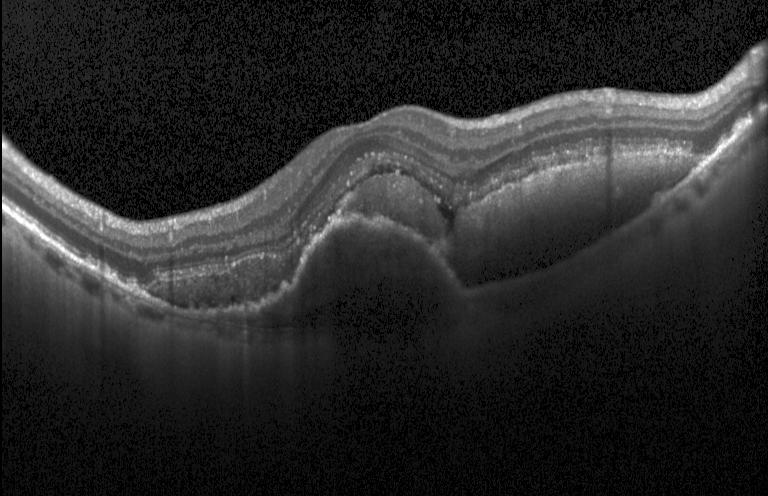 Spectral-domain optical coherence tomography; Heidelberg Spectralis; fovea-centered; optical coherence tomography scan — Diagnosis: a choroidal neovascular membrane.